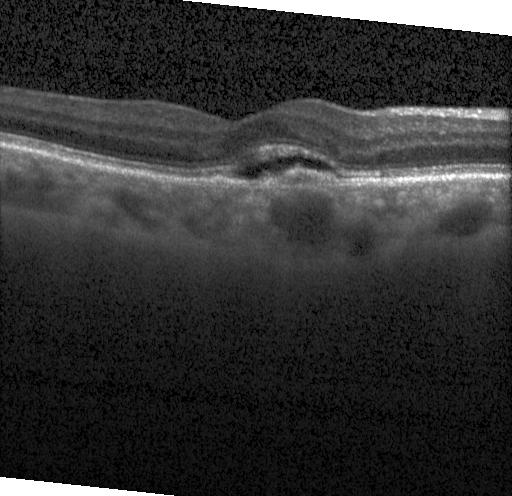 Dx: a choroidal neovascular membrane.